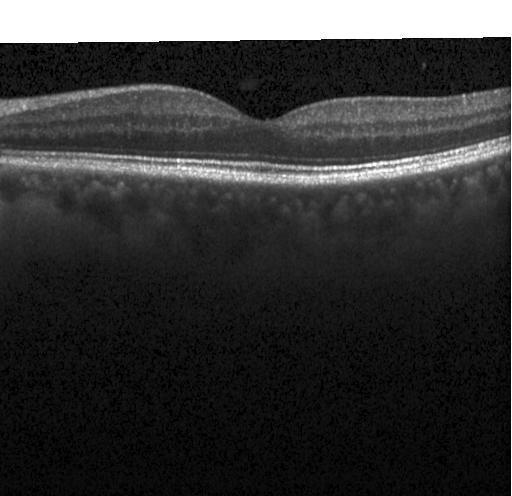

This B-scan demonstrates no evidence of choroidal neovascularization, diabetic macular edema, or drusen.